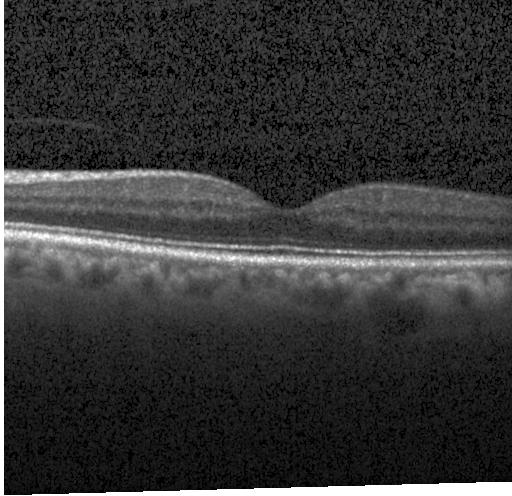 Dx: neither choroidal neovascularization, diabetic macular edema, nor drusen.